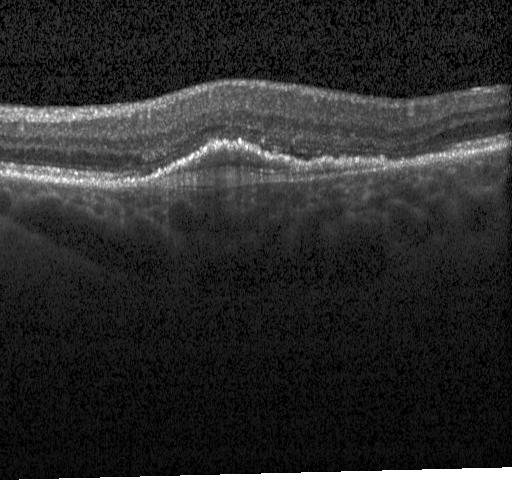

OCT scan showing choroidal neovascularization (CNV).